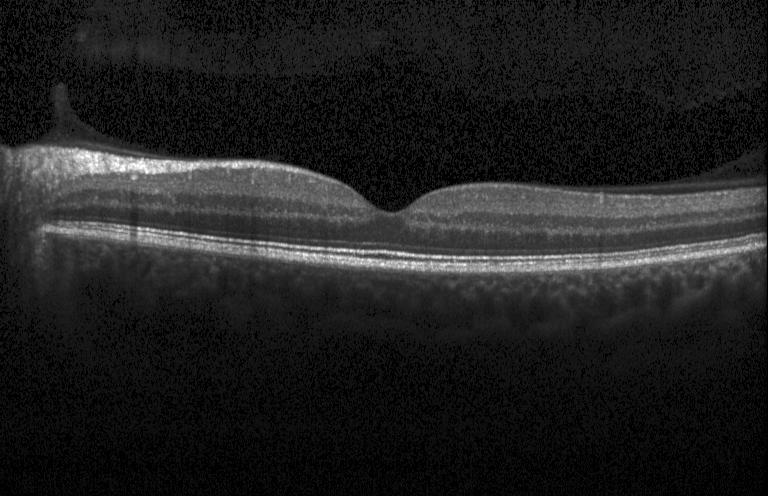

Diagnosis: no choroidal neovascularization, diabetic macular edema, or drusen.